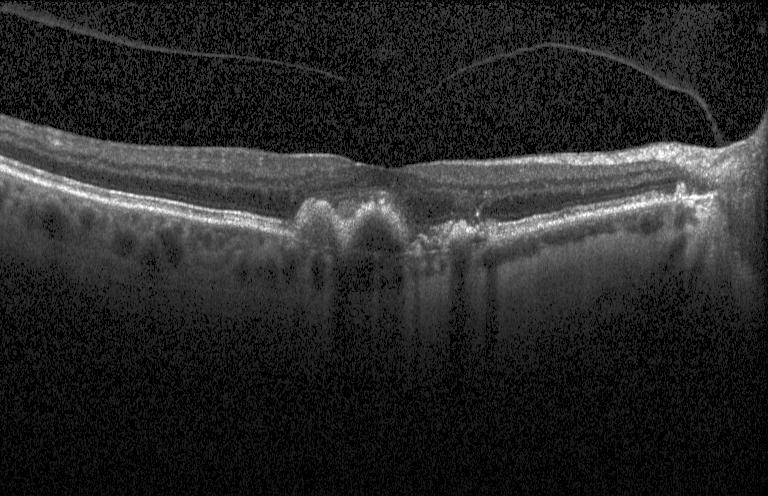 CNV.